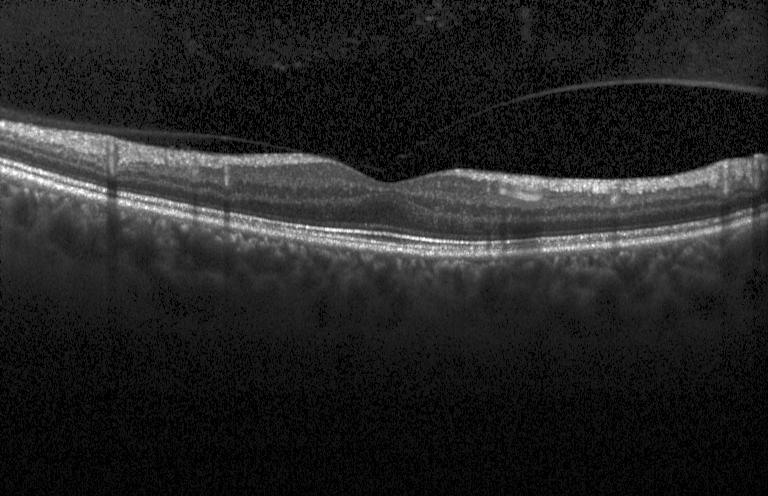 The scan shows no choroidal neovascularization, diabetic macular edema, or drusen.